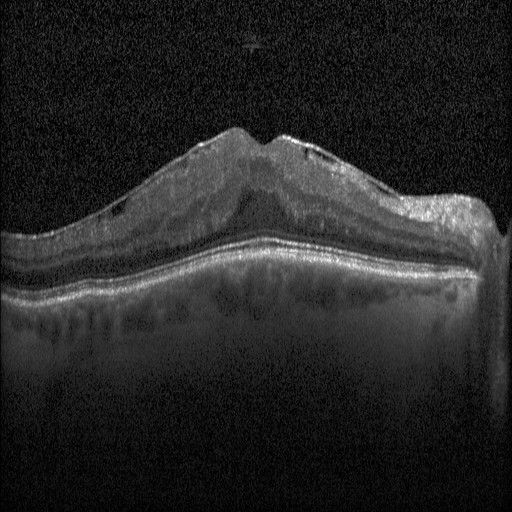
Macular OCT demonstrating DME.